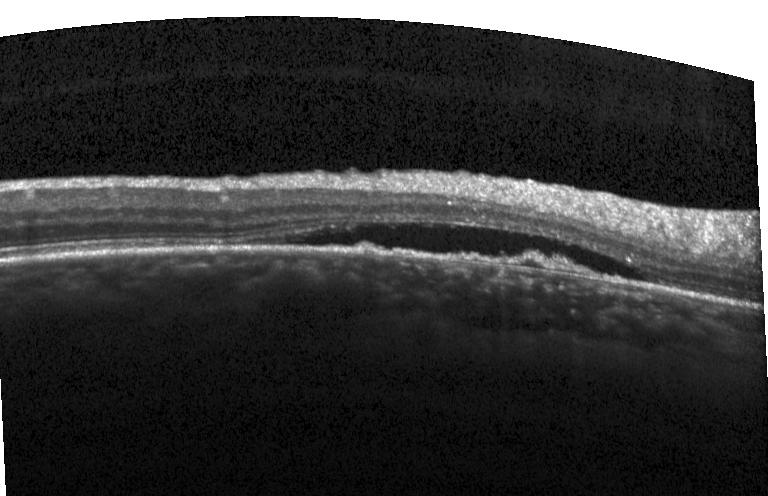

OCT B-scan — This B-scan demonstrates a choroidal neovascular membrane.